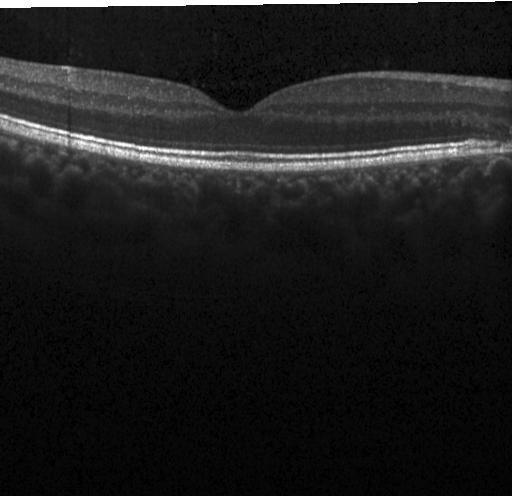

OCT finding: neither CNV, DME, nor drusen.